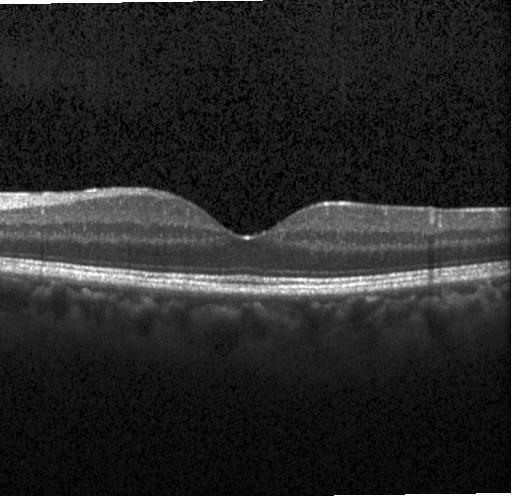

Optical coherence tomography scan. Instrument: Heidelberg Spectralis — Assessment: no evidence of choroidal neovascularization, diabetic macular edema, or drusen.